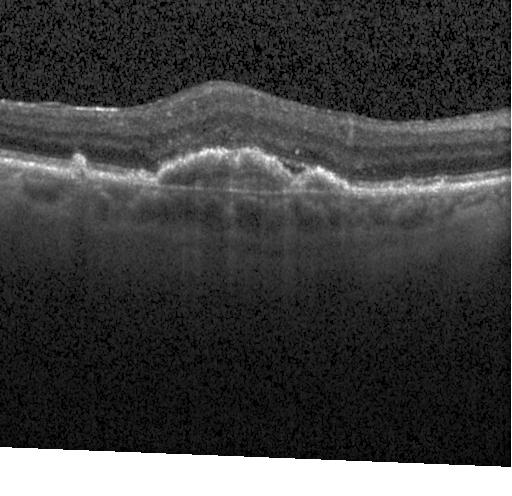 Horizontal scan through the fovea, retinal OCT cross-section. Impression: a choroidal neovascular membrane.